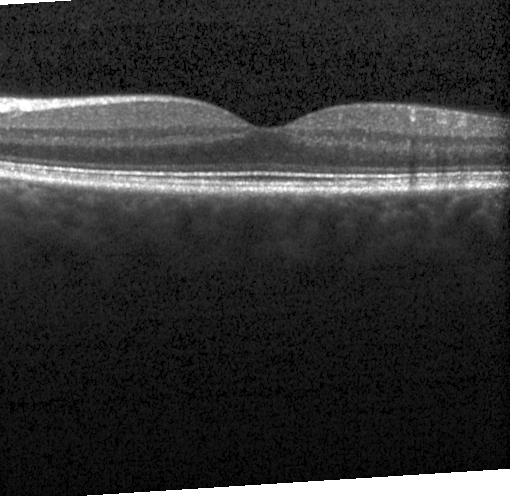 Macular OCT: no evidence of choroidal neovascularization, diabetic macular edema, or drusen.